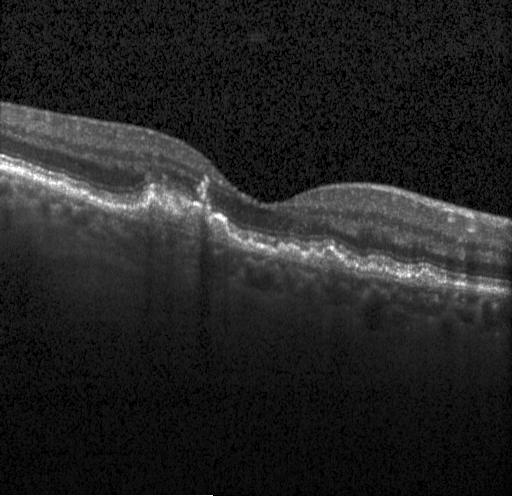 Horizontal scan through the fovea; retinal OCT cross-section; Heidelberg Spectralis OCT system — The scan shows choroidal neovascularization (CNV).